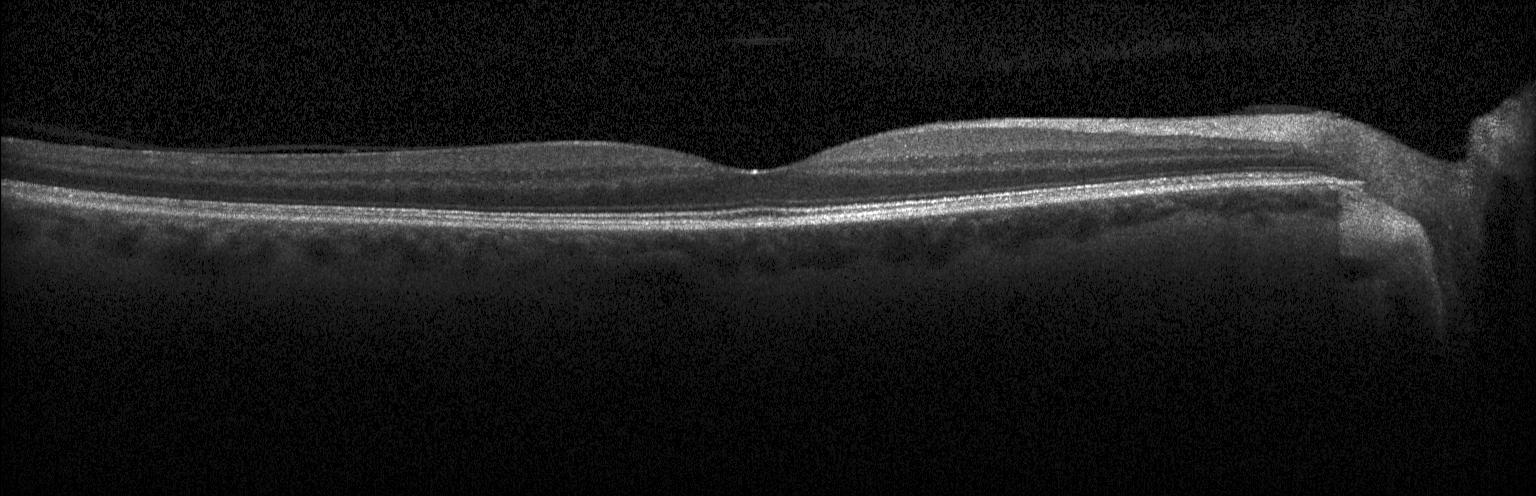 Through the macula · Heidelberg Spectralis · retinal OCT cross-section · spectral-domain optical coherence tomography — The scan shows no choroidal neovascularization, diabetic macular edema, or drusen.